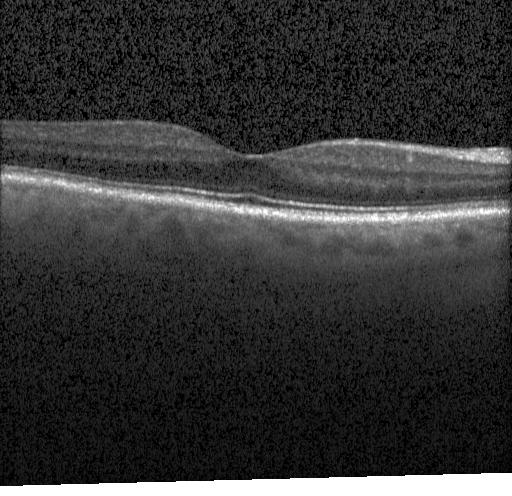
This B-scan demonstrates no choroidal neovascularization, diabetic macular edema, or drusen.